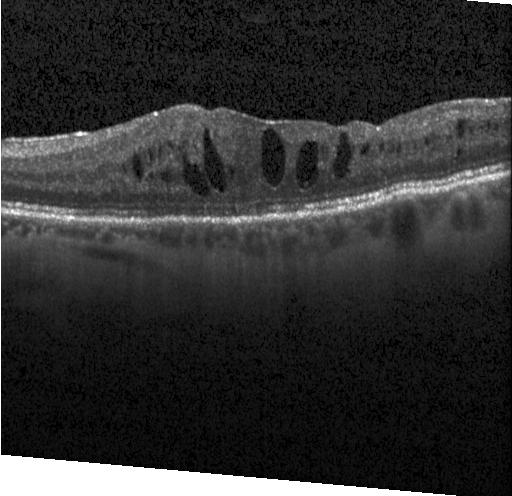

Finding: diabetic macular edema (DME).